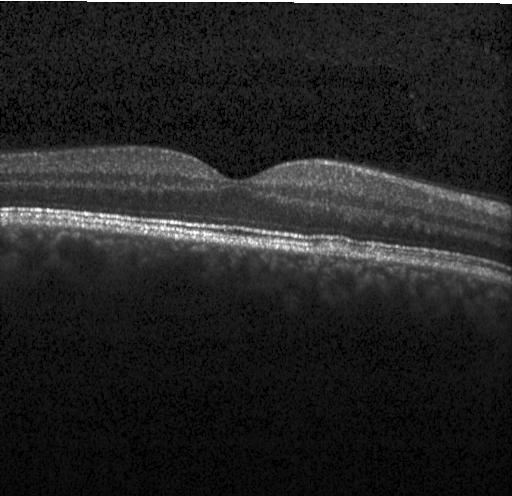 Macular OCT: no choroidal neovascularization, no diabetic macular edema, and no drusen.